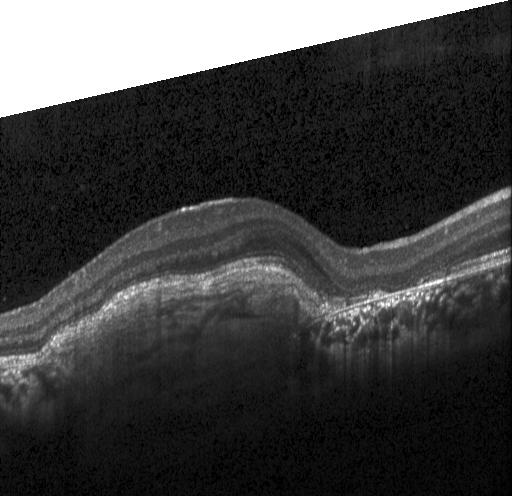

Optical coherence tomography scan.
Impression: CNV.